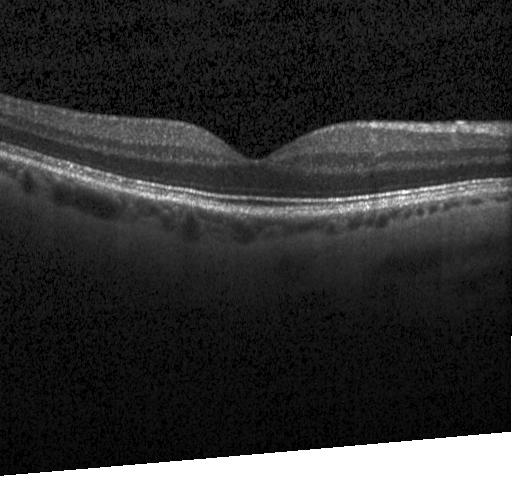 OCT line scan. Macular OCT: no choroidal neovascularization, no diabetic macular edema, and no drusen.